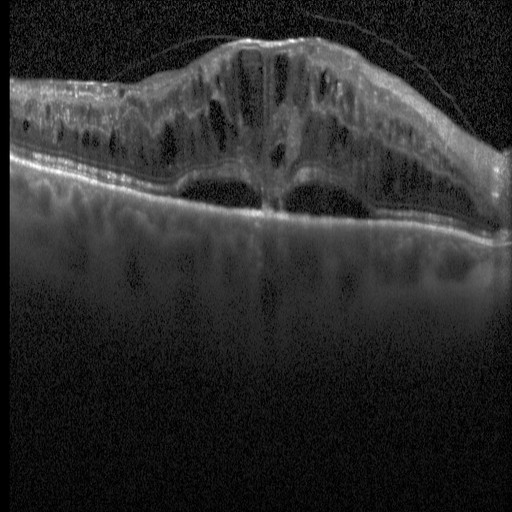
OCT line scan. Impression: diabetic macular edema.